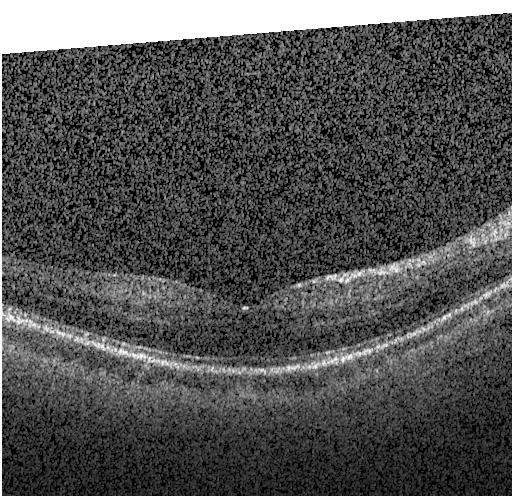

Dx: no choroidal neovascularization, no diabetic macular edema, and no drusen.